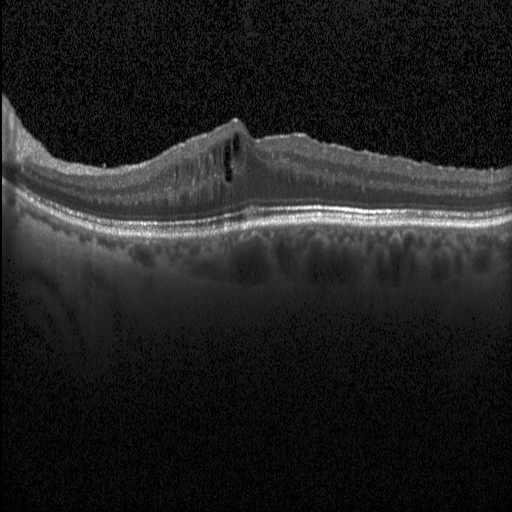

Optical coherence tomography scan, Heidelberg Spectralis OCT system, SD-OCT
OCT finding: DME.